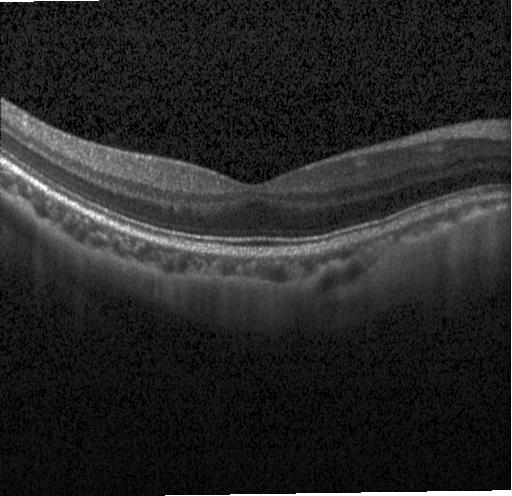 Through the macula, OCT line scan, Heidelberg Spectralis. Assessment: no evidence of choroidal neovascularization, diabetic macular edema, or drusen.